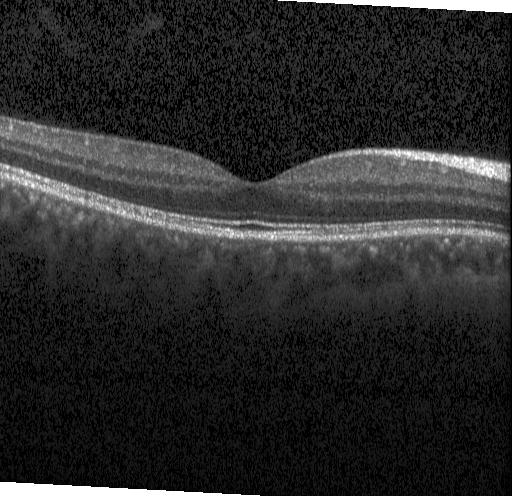 Finding: no choroidal neovascularization, no diabetic macular edema, and no drusen.